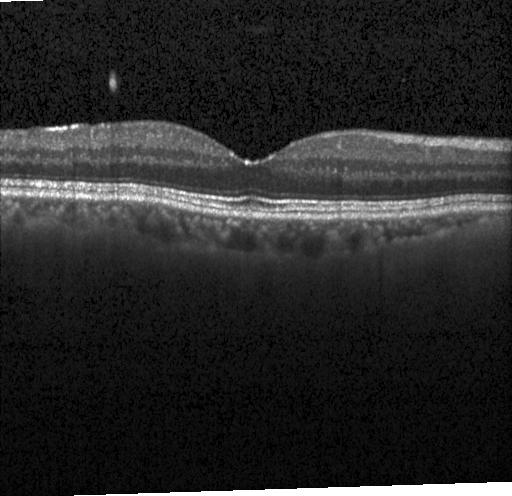
OCT scan showing no choroidal neovascularization, diabetic macular edema, or drusen.